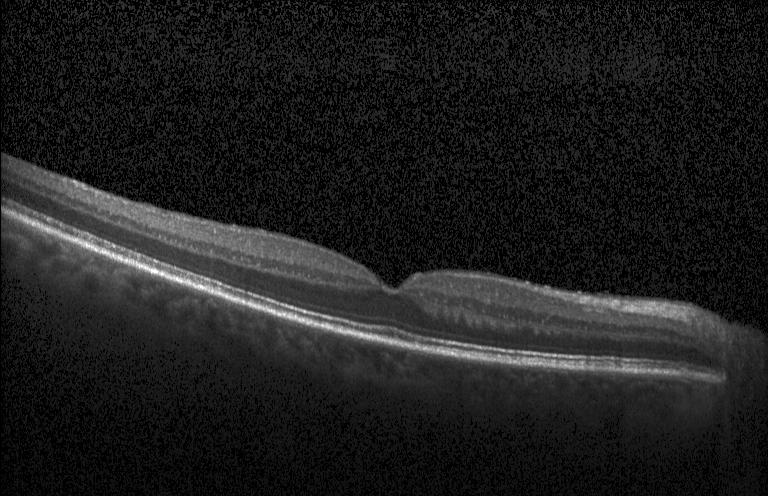 Spectral-domain OCT, Heidelberg Spectralis OCT system, retinal OCT cross-section. No evidence of choroidal neovascularization, diabetic macular edema, or drusen.